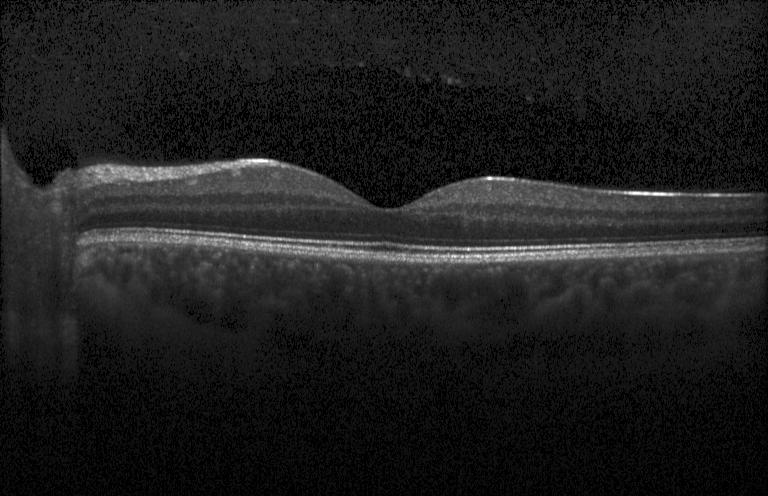 Macular scan · SD-OCT · OCT line scan · Heidelberg Spectralis. OCT finding: neither CNV, DME, nor drusen.